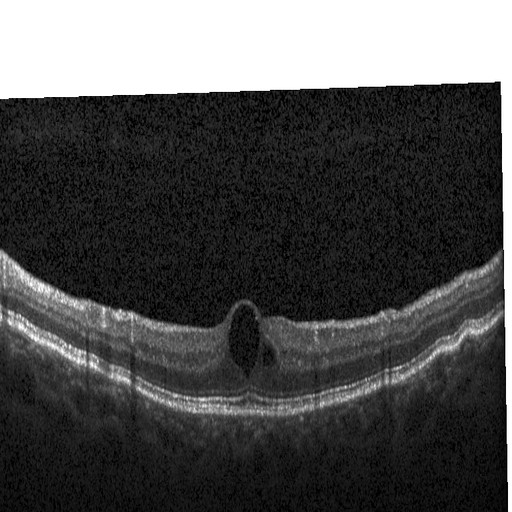
Instrument: Heidelberg Spectralis; spectral-domain optical coherence tomography; OCT B-scan; through the macula — The scan shows diabetic macular edema (DME).